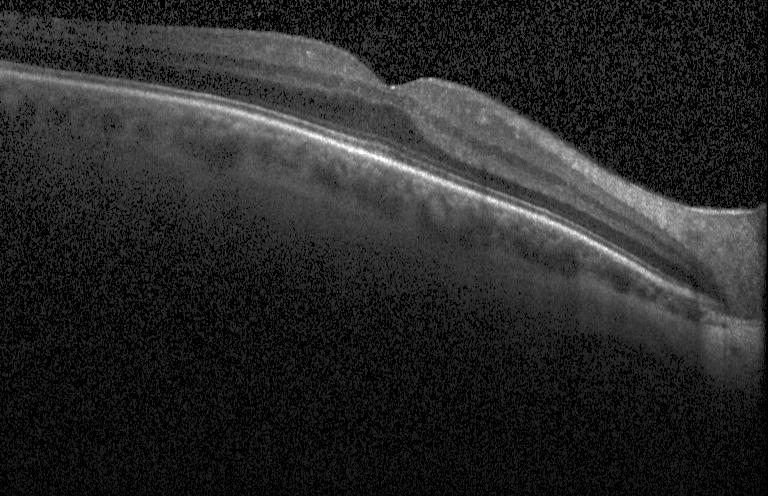

Spectral-domain OCT. Heidelberg Spectralis OCT system. Retinal OCT cross-section. Dx: neither choroidal neovascularization, diabetic macular edema, nor drusen.